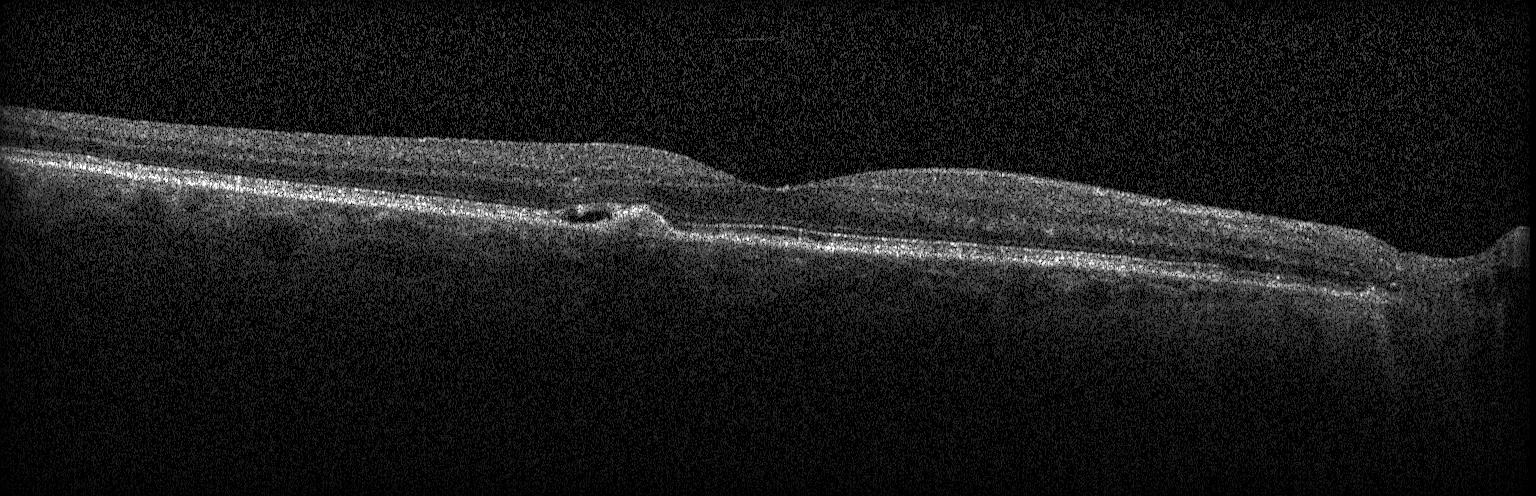
CNV.